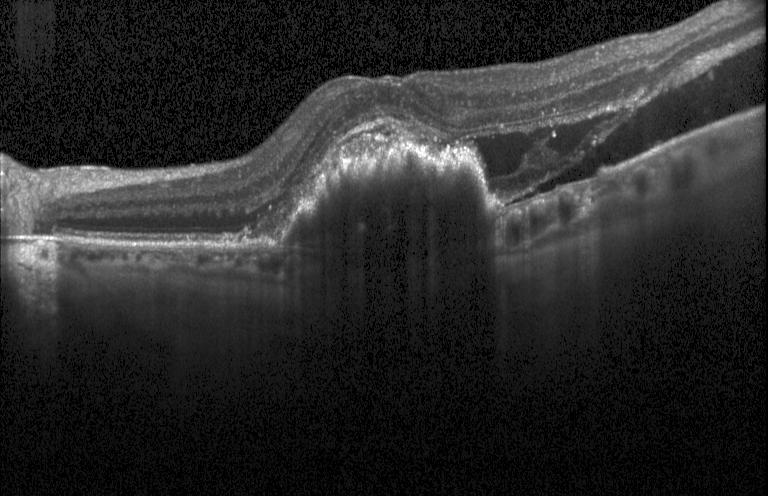

Spectral-domain OCT · Heidelberg Spectralis OCT system · centered on the fovea · optical coherence tomography scan — Dx: a choroidal neovascular membrane.